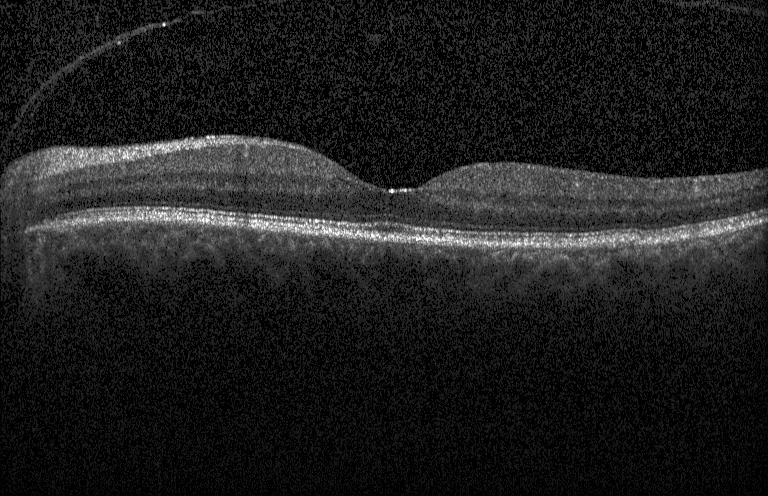

Centered on the fovea, Heidelberg Spectralis, spectral-domain OCT, retinal OCT B-scan. Finding: no evidence of choroidal neovascularization, diabetic macular edema, or drusen.